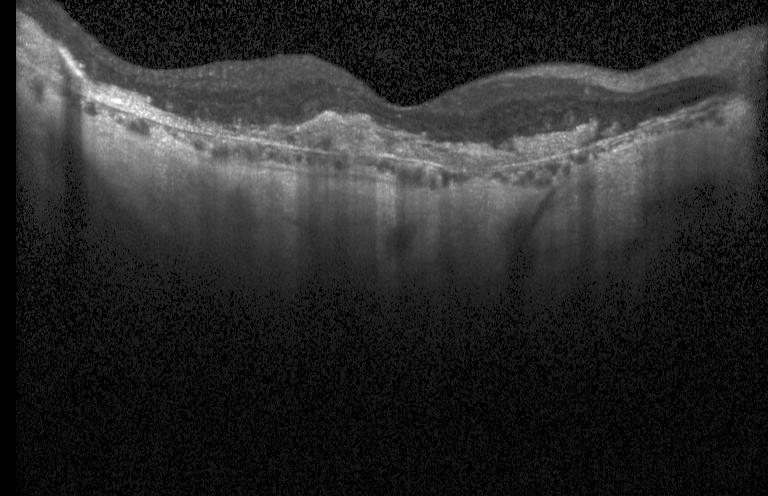
Macular OCT demonstrating choroidal neovascularization (CNV).